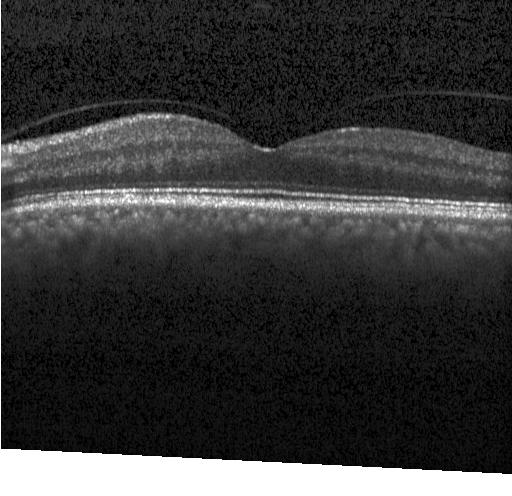

Heidelberg Spectralis, fovea-centered, retinal OCT B-scan — Diagnosis: no choroidal neovascularization, diabetic macular edema, or drusen.